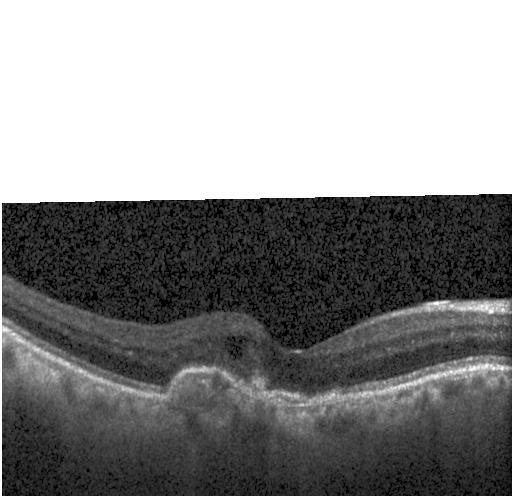 Spectral-domain optical coherence tomography; through the macula; retinal OCT B-scan
Macular OCT: choroidal neovascularization (CNV).